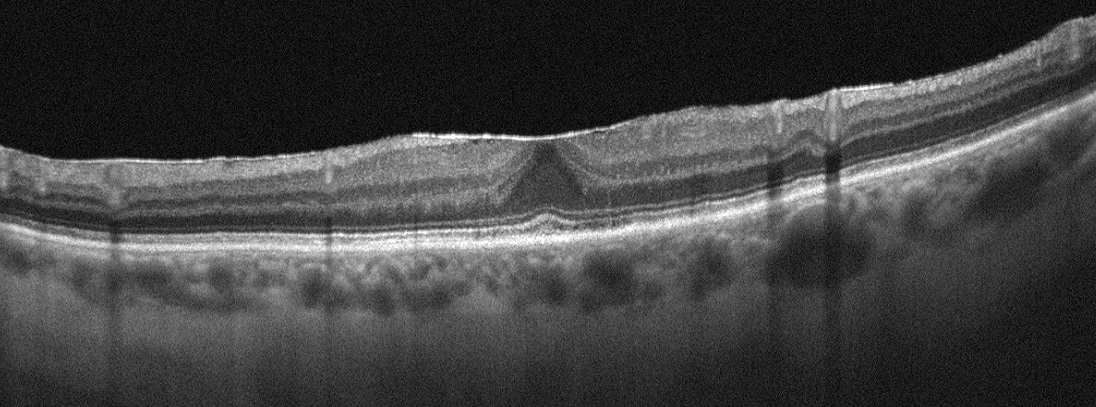 Retinal OCT B-scan
Assessment: epiretinal membrane.